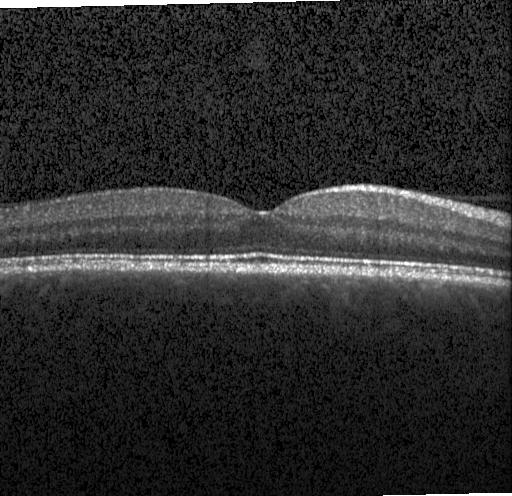

Impression: neither choroidal neovascularization, diabetic macular edema, nor drusen.